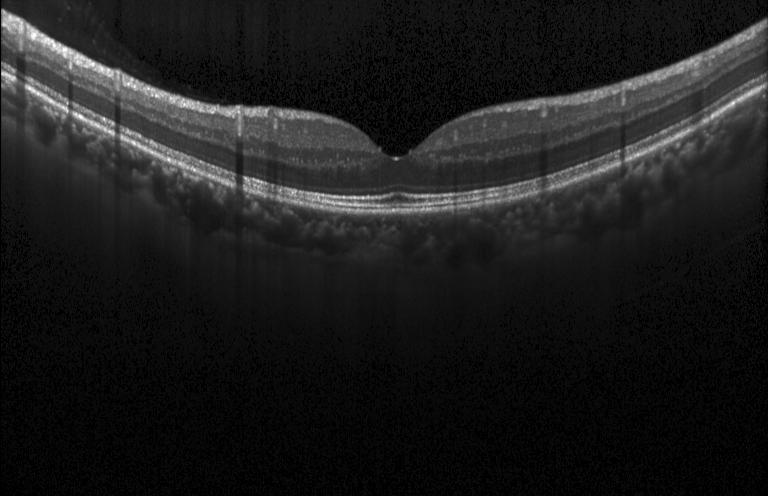

Dx: neither CNV, DME, nor drusen.